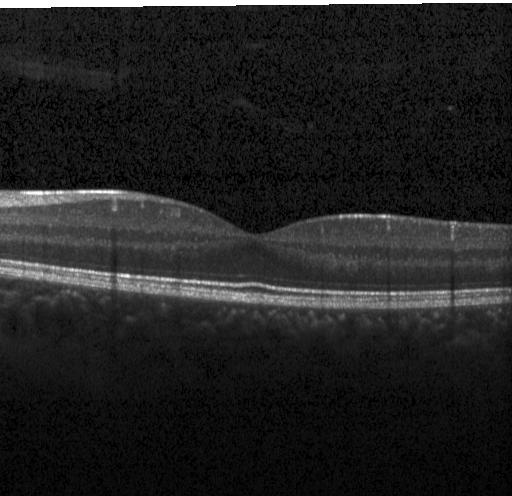

Retinal OCT B-scan — Finding: neither choroidal neovascularization, diabetic macular edema, nor drusen.